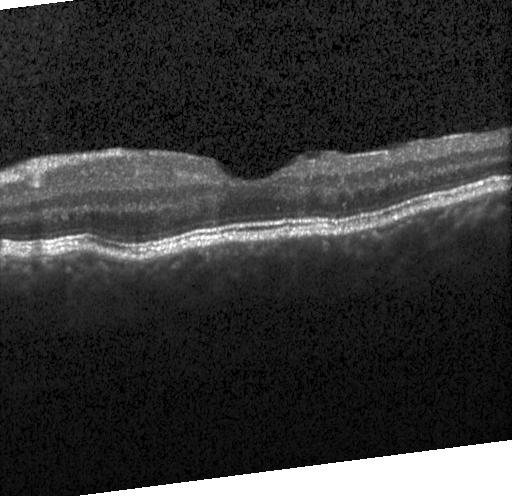 Instrument: Heidelberg Spectralis; retinal OCT cross-section. Dx: no choroidal neovascularization, diabetic macular edema, or drusen.